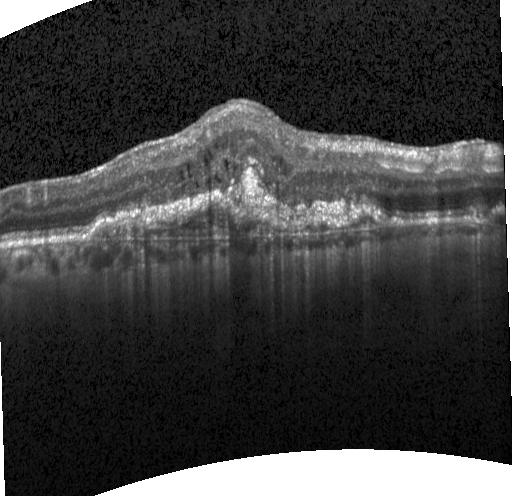
Optical coherence tomography B-scan · spectral-domain OCT. The scan shows CNV.